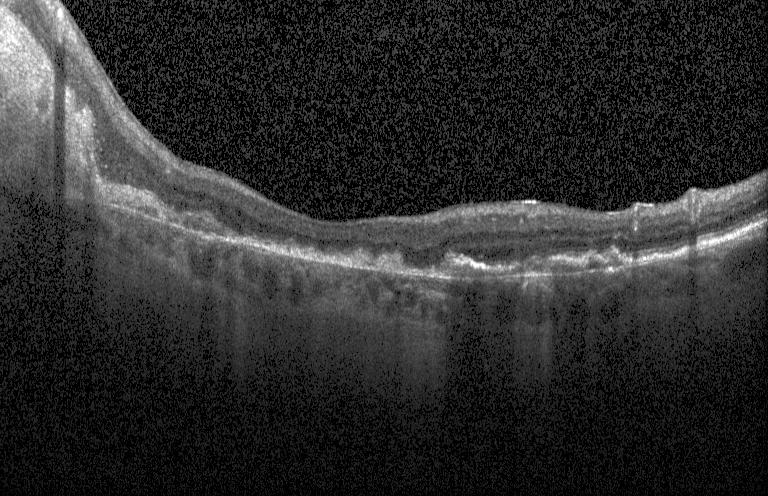 Impression: choroidal neovascularization.